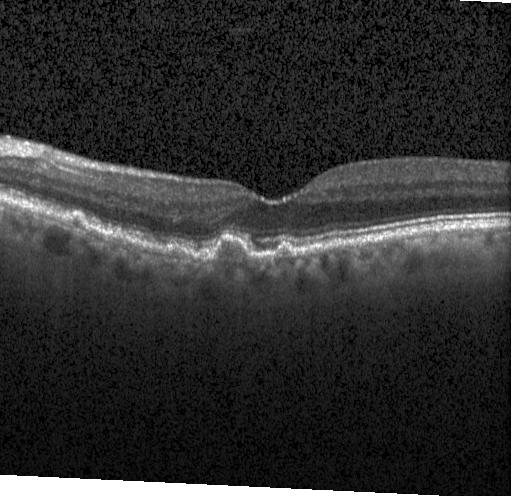
Spectral-domain OCT, optical coherence tomography scan
OCT finding: drusen.